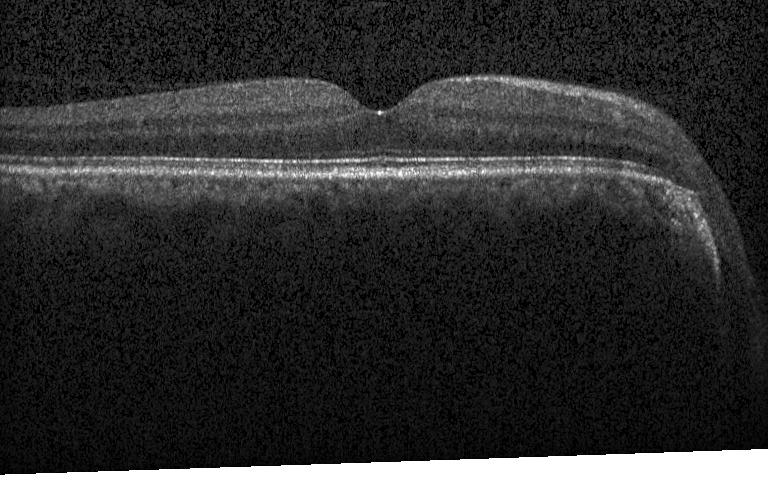

OCT finding: neither choroidal neovascularization, diabetic macular edema, nor drusen.